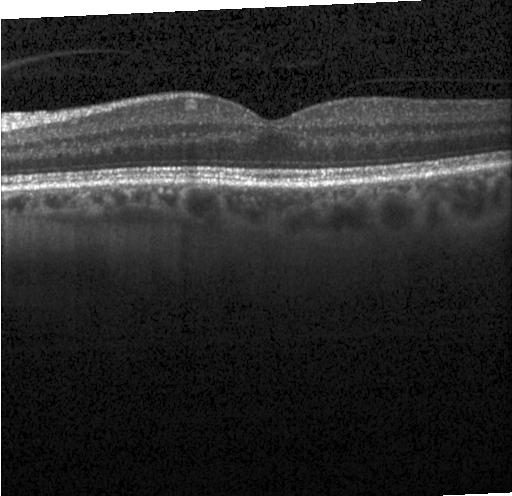
Retinal OCT B-scan.
Dx: no evidence of CNV, DME, or drusen.